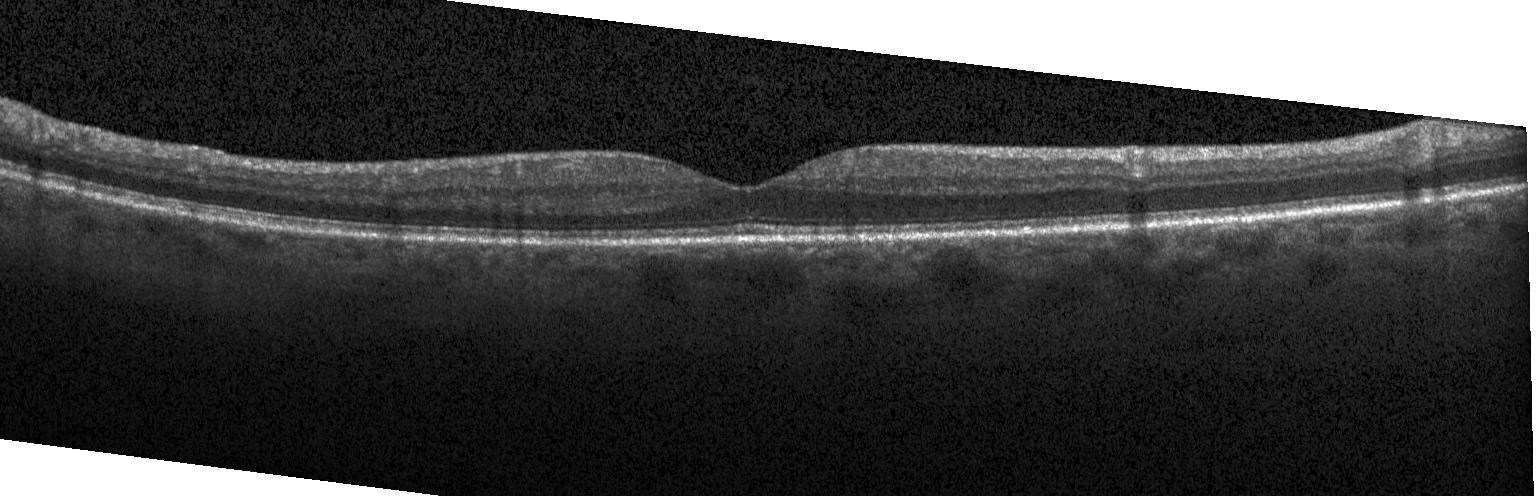 Optical coherence tomography B-scan; acquired on a Heidelberg Spectralis — Macular OCT: no choroidal neovascularization, no diabetic macular edema, and no drusen.